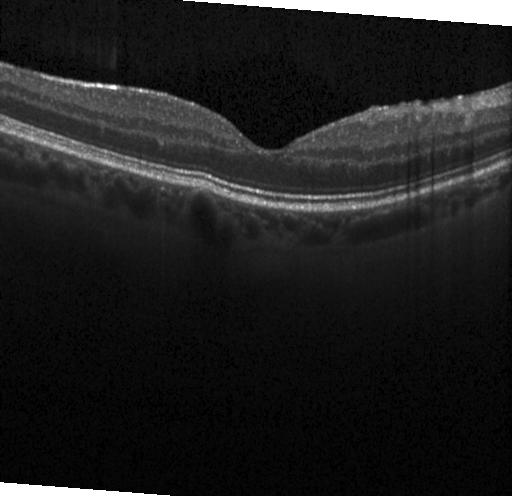
Fovea-centered; OCT line scan; spectral-domain optical coherence tomography
Diagnosis: no choroidal neovascularization, diabetic macular edema, or drusen.